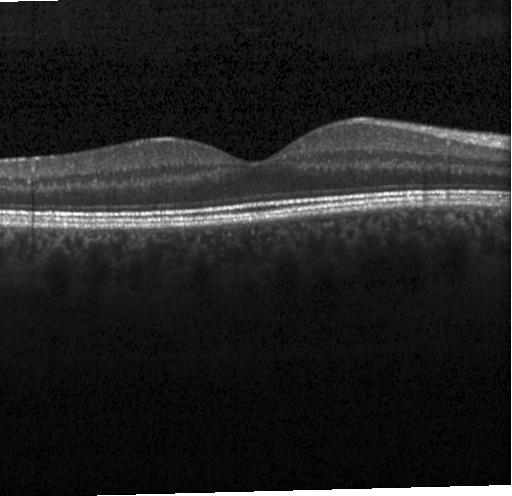
OCT B-scan showing neither choroidal neovascularization, diabetic macular edema, nor drusen.